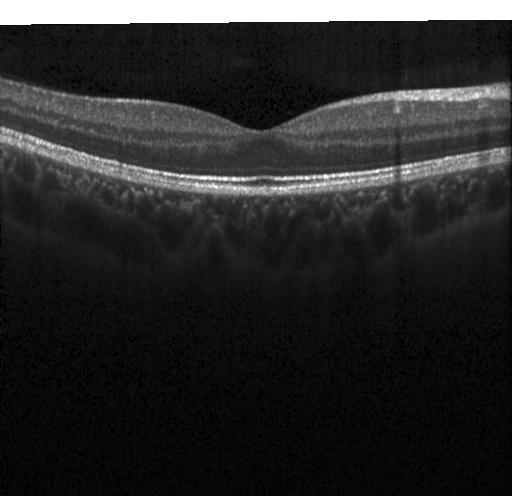 Optical coherence tomography scan
Macular OCT: no evidence of CNV, DME, or drusen.